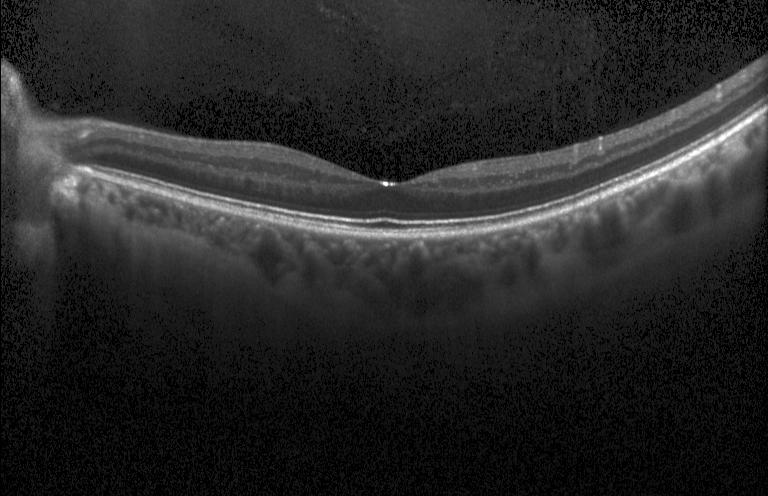
Spectral-domain optical coherence tomography, retinal OCT B-scan — Macular OCT: neither choroidal neovascularization, diabetic macular edema, nor drusen.